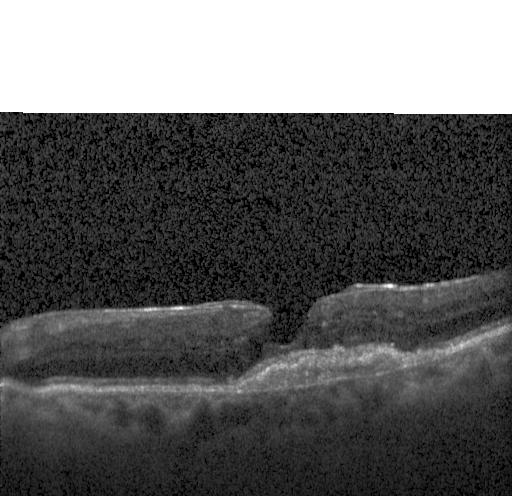 Dx: CNV.